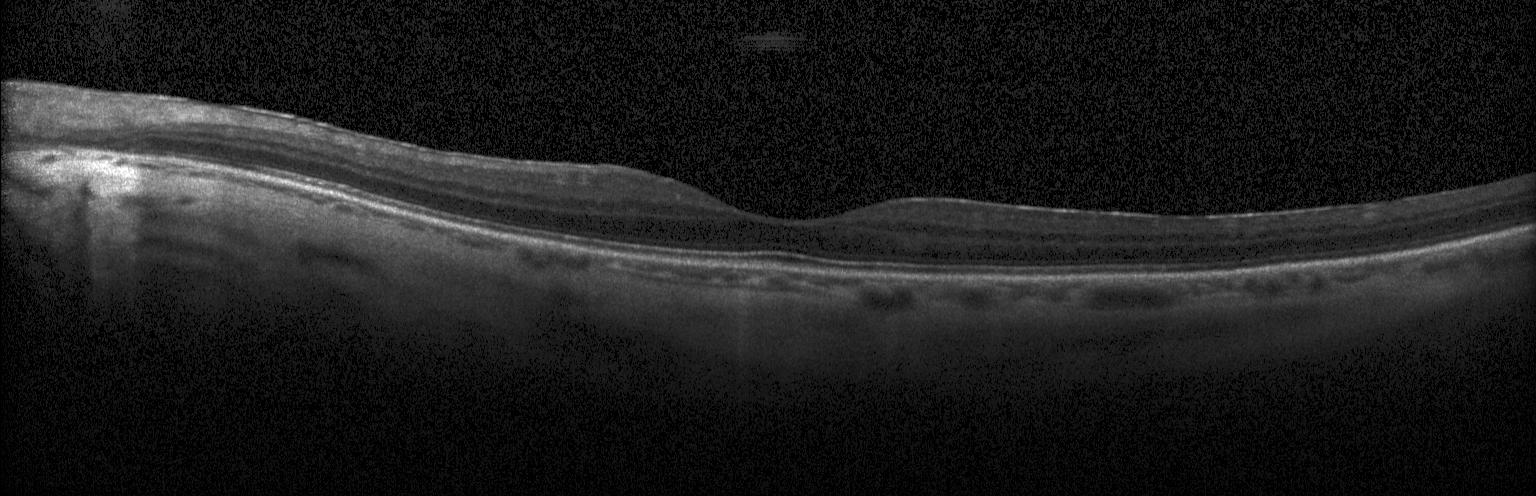 Spectral-domain OCT; optical coherence tomography B-scan. Finding: neither choroidal neovascularization, diabetic macular edema, nor drusen.